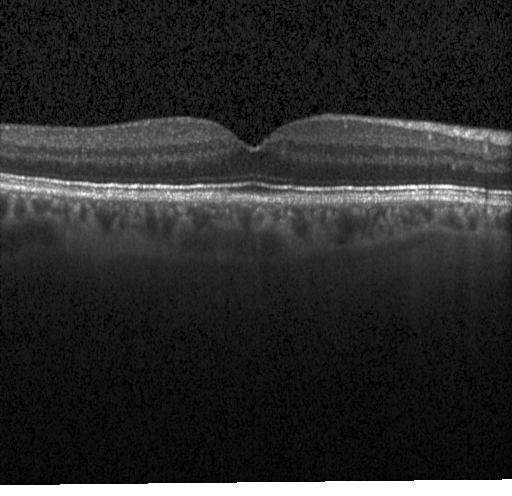
Diagnosis: neither choroidal neovascularization, diabetic macular edema, nor drusen.